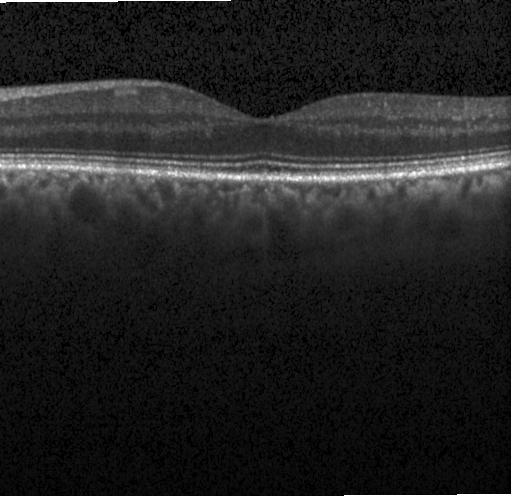 Heidelberg Spectralis; through the macula; spectral-domain optical coherence tomography; retinal OCT B-scan. Assessment: neither CNV, DME, nor drusen.